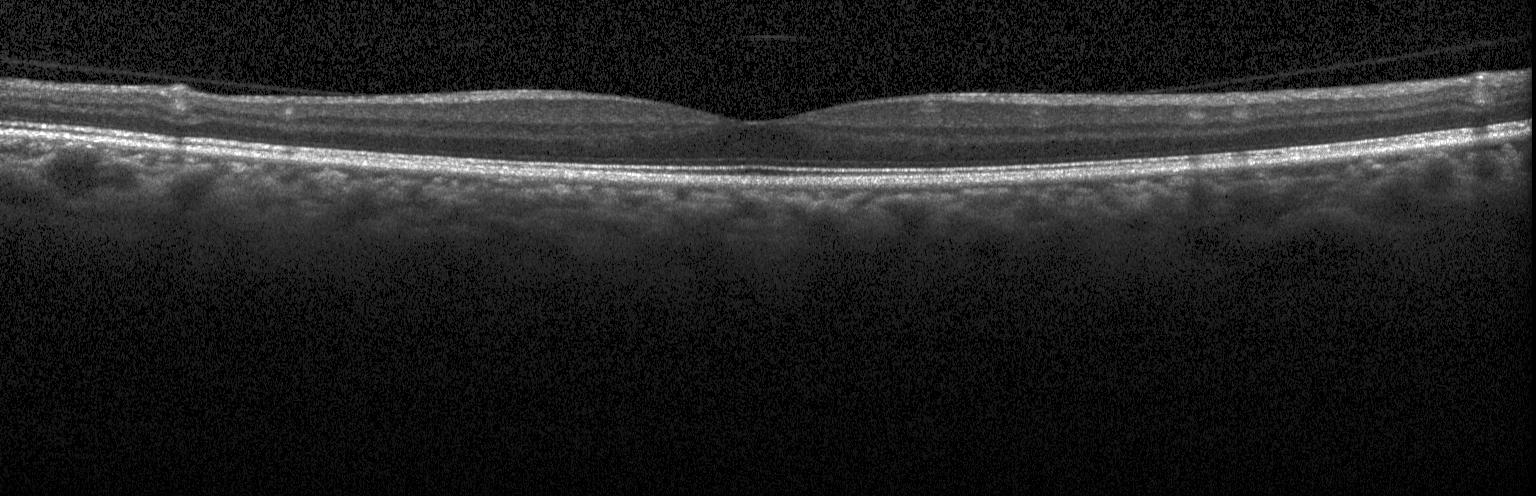 Macular OCT: neither CNV, DME, nor drusen.